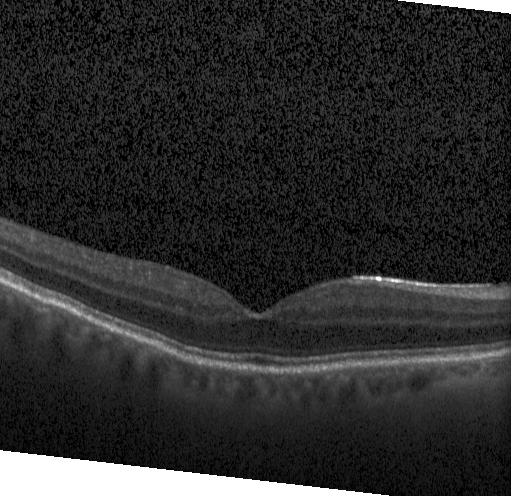
Retinal OCT B-scan; acquired on a Heidelberg Spectralis; macular scan; spectral-domain optical coherence tomography
Dx: no evidence of choroidal neovascularization, diabetic macular edema, or drusen.